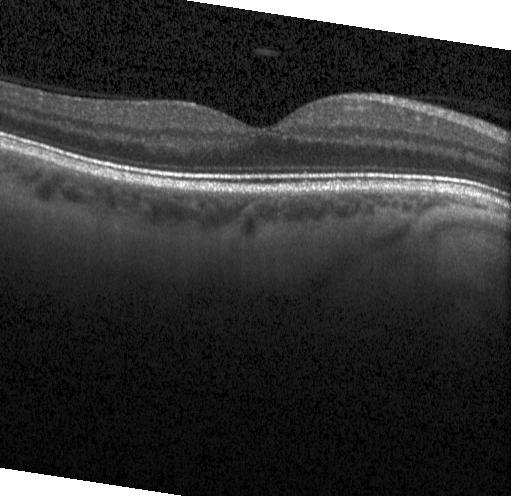

Horizontal scan through the fovea; acquired on a Heidelberg Spectralis; SD-OCT; optical coherence tomography B-scan.
Dx: no evidence of CNV, DME, or drusen.